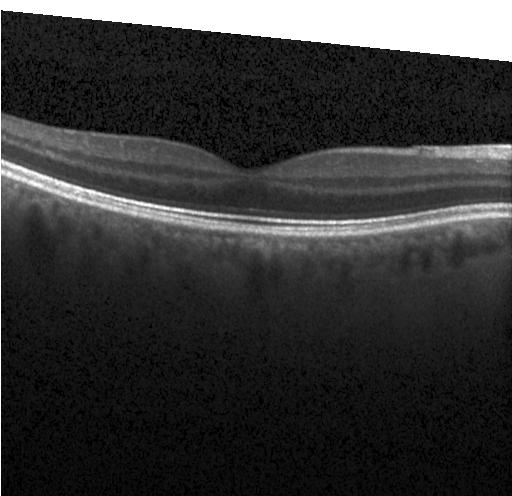

Spectral-domain OCT · optical coherence tomography scan · macular scan — Finding: no choroidal neovascularization, no diabetic macular edema, and no drusen.